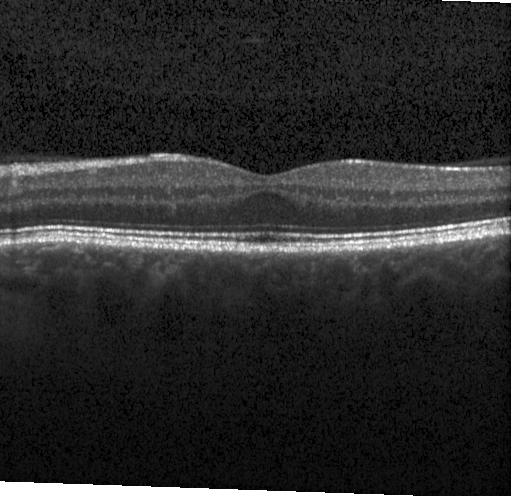 Retinal OCT cross-section. No choroidal neovascularization, diabetic macular edema, or drusen.